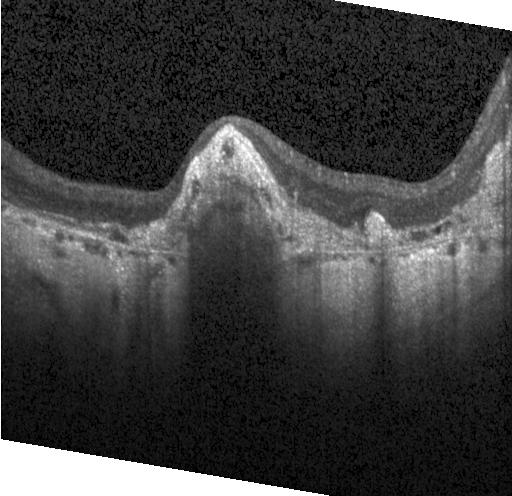
Dx: choroidal neovascularization.